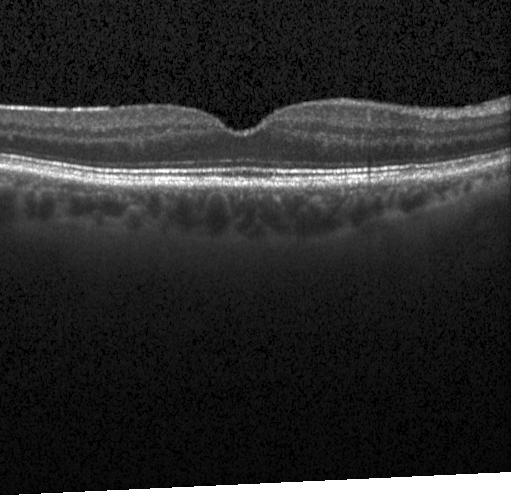

Retinal OCT B-scan, spectral-domain OCT, Heidelberg Spectralis, centered on the fovea. Impression: no evidence of CNV, DME, or drusen.